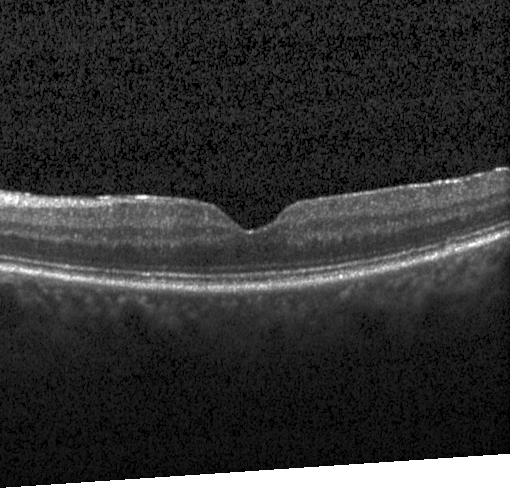 Macular OCT: no CNV, DME, or drusen.